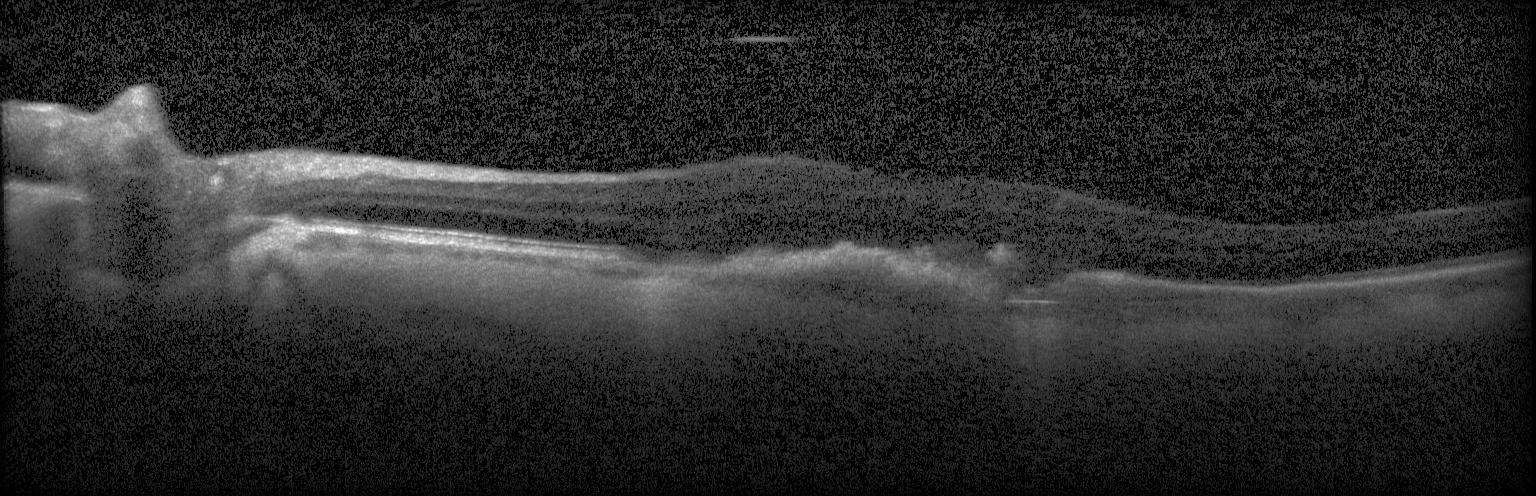
SD-OCT · optical coherence tomography scan.
Assessment: choroidal neovascularization (CNV).